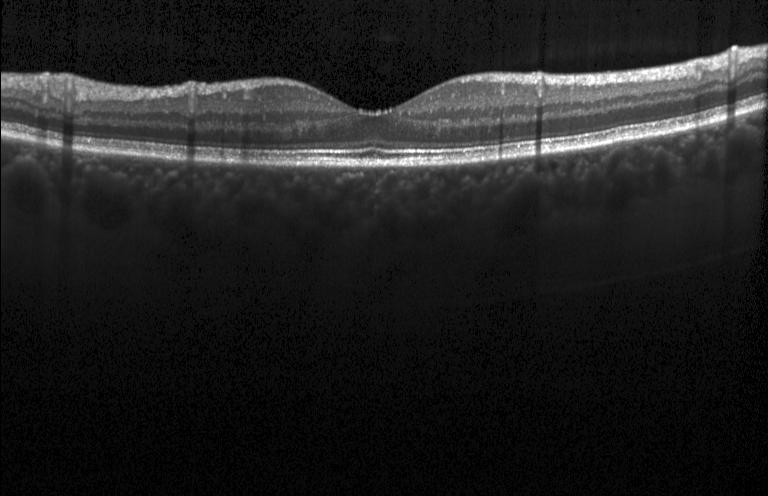 Macular OCT: no CNV, DME, or drusen.